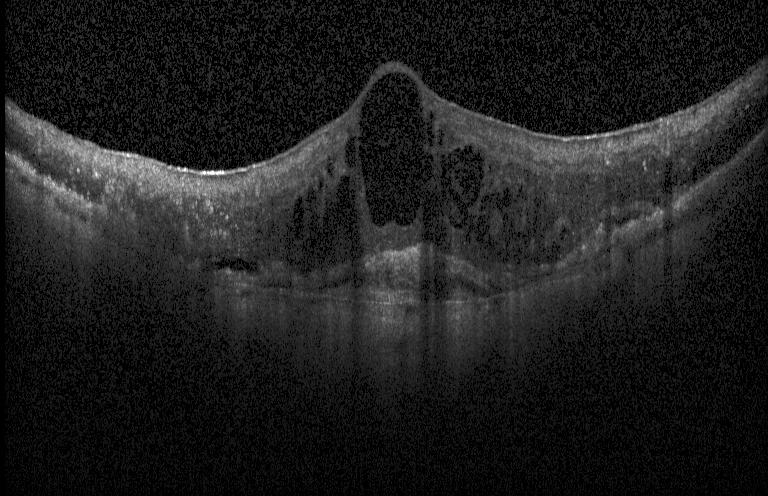

OCT finding: a choroidal neovascular membrane.